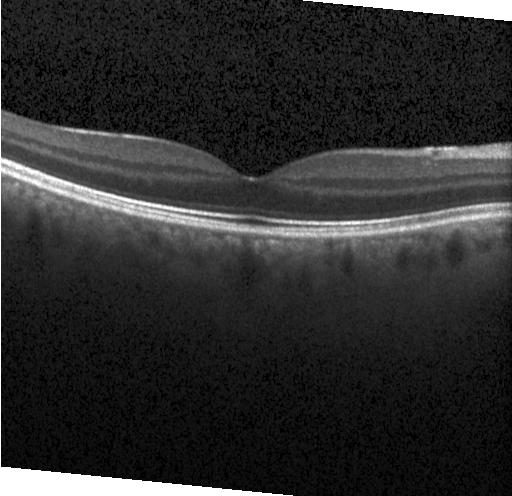 Assessment: no choroidal neovascularization, diabetic macular edema, or drusen.